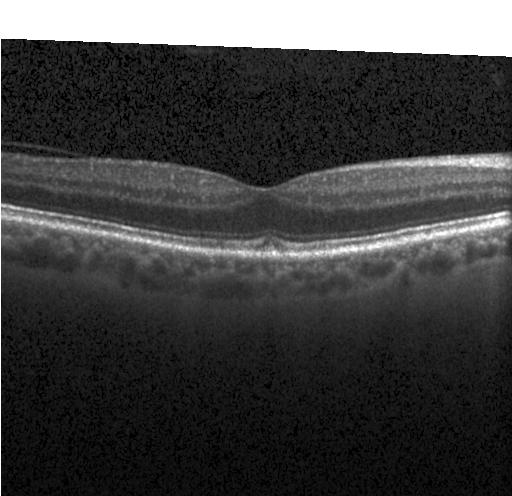 Impression: no choroidal neovascularization, diabetic macular edema, or drusen.